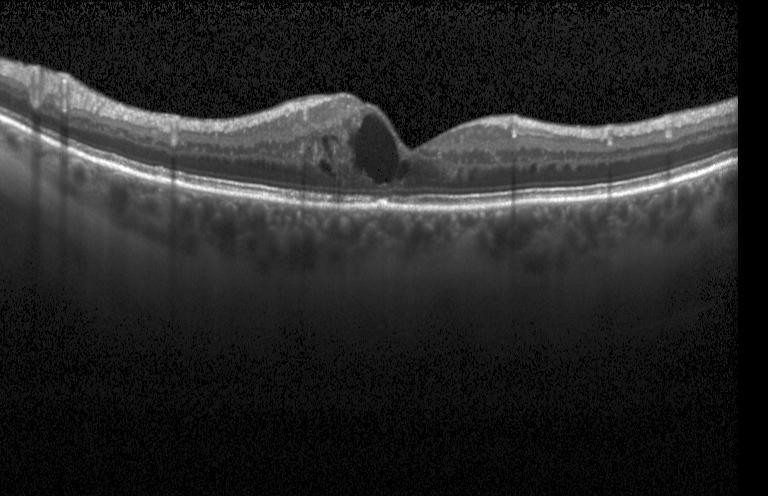

The scan shows diabetic macular edema.